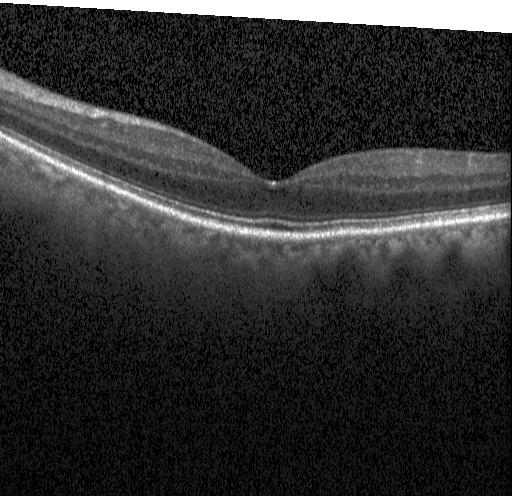

Instrument: Heidelberg Spectralis · OCT B-scan · centered on the fovea.
Finding: no CNV, DME, or drusen.